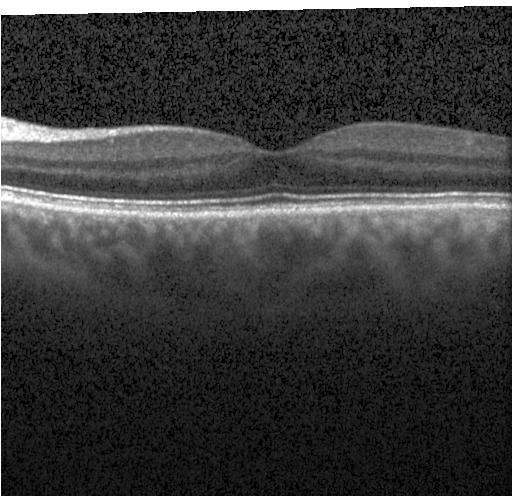

Acquired on a Heidelberg Spectralis; spectral-domain OCT; retinal OCT cross-section. Impression: no CNV, DME, or drusen.